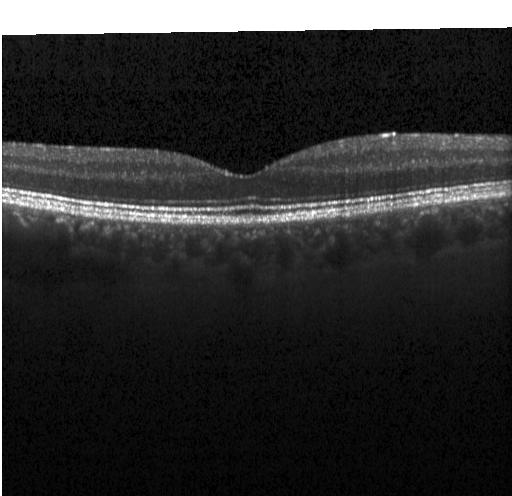

No evidence of choroidal neovascularization, diabetic macular edema, or drusen.